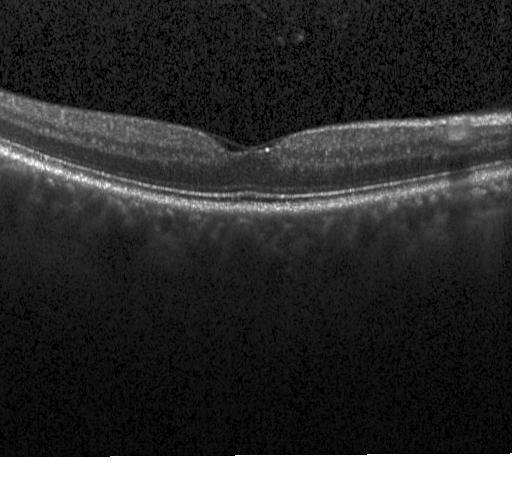
Retinal OCT cross-section, centered on the fovea
Finding: no evidence of choroidal neovascularization, diabetic macular edema, or drusen.